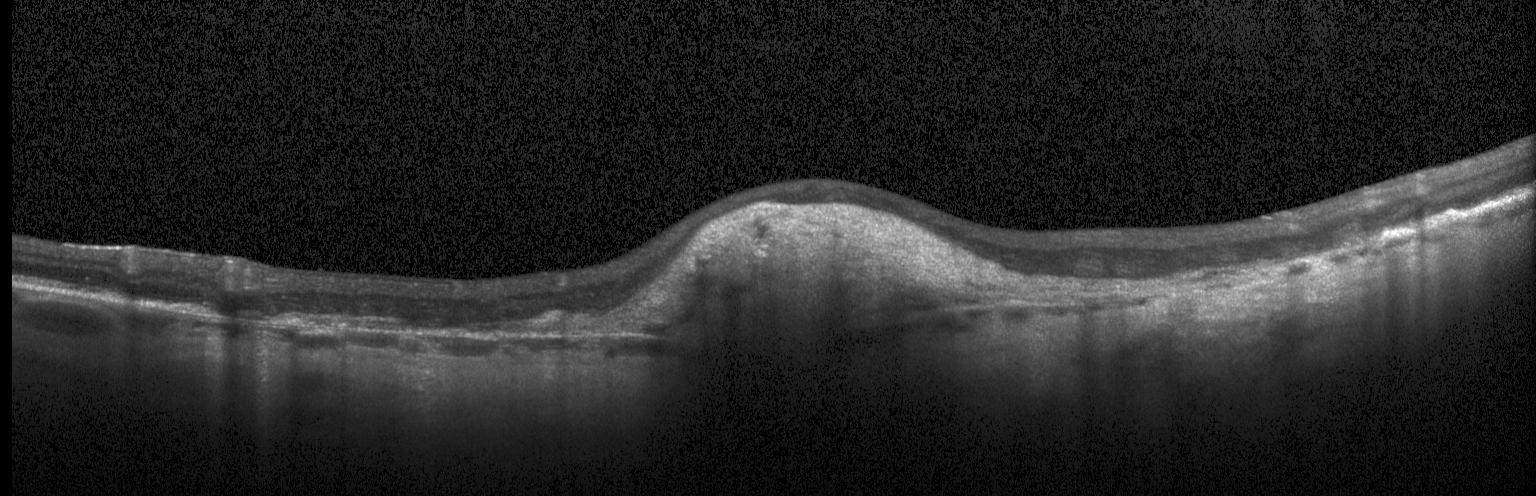

Through the macula. Optical coherence tomography B-scan.
The scan shows CNV.